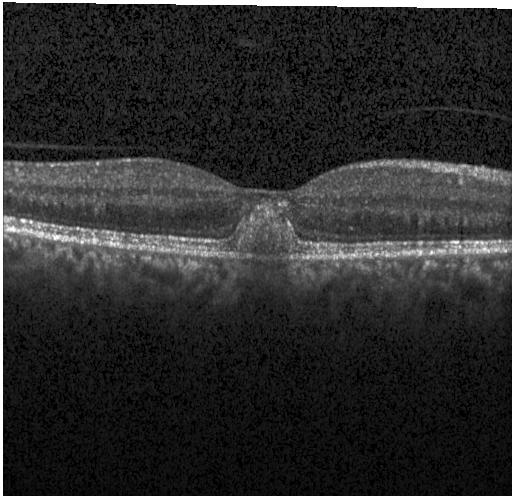 OCT scan showing CNV.